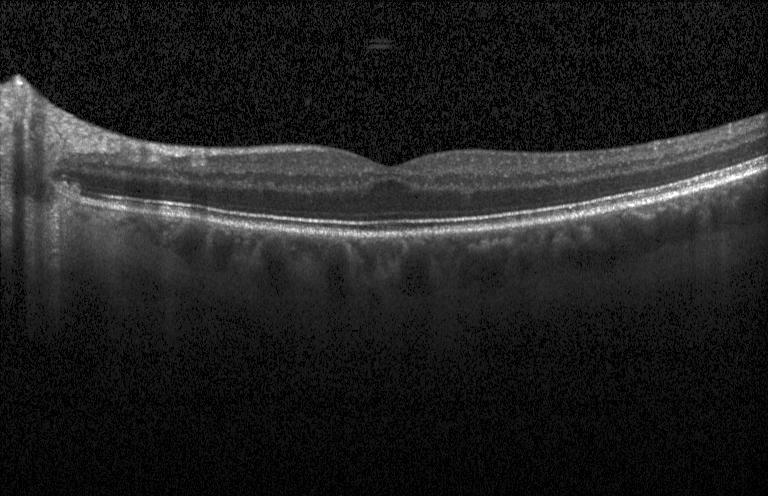
Diagnosis: no choroidal neovascularization, no diabetic macular edema, and no drusen.